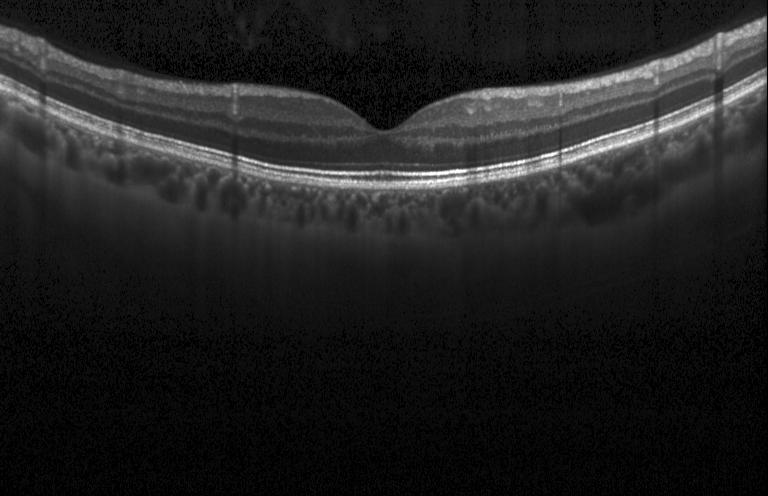

Retinal OCT B-scan.
No evidence of choroidal neovascularization, diabetic macular edema, or drusen.